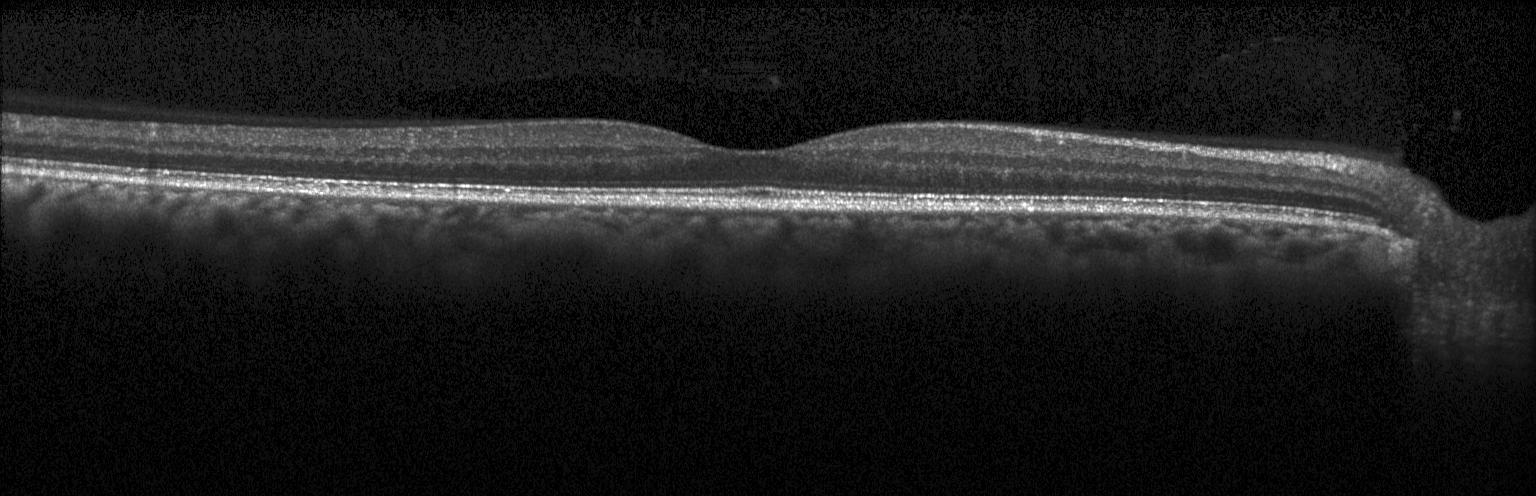

Centered on the fovea · SD-OCT · retinal OCT cross-section · Heidelberg Spectralis OCT system. Assessment: no choroidal neovascularization, diabetic macular edema, or drusen.